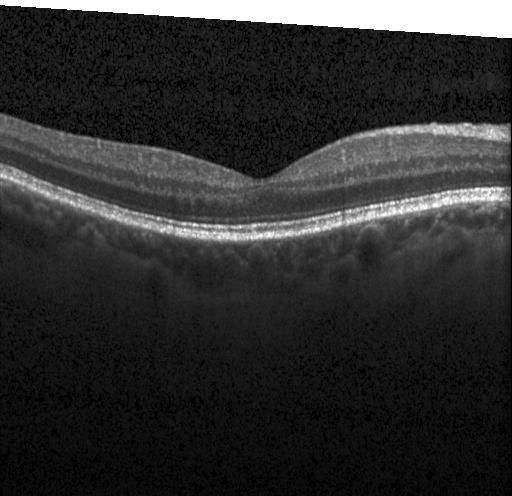

Optical coherence tomography B-scan · acquired on a Heidelberg Spectralis · spectral-domain OCT — No choroidal neovascularization, no diabetic macular edema, and no drusen.